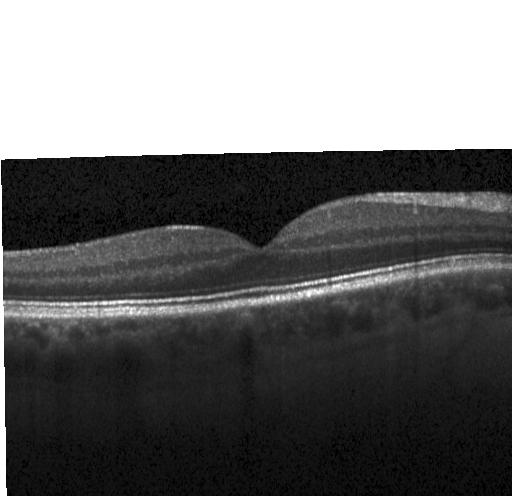
Macular OCT: no choroidal neovascularization, no diabetic macular edema, and no drusen.